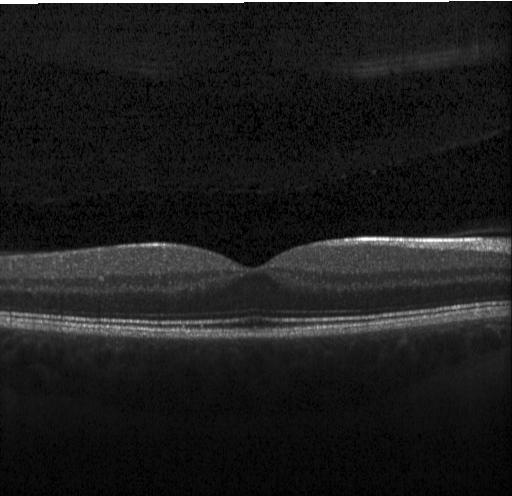

Diagnosis: no choroidal neovascularization, no diabetic macular edema, and no drusen.